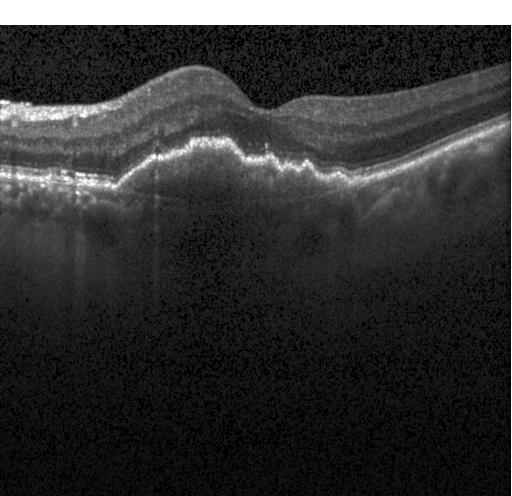
OCT scan showing choroidal neovascularization.